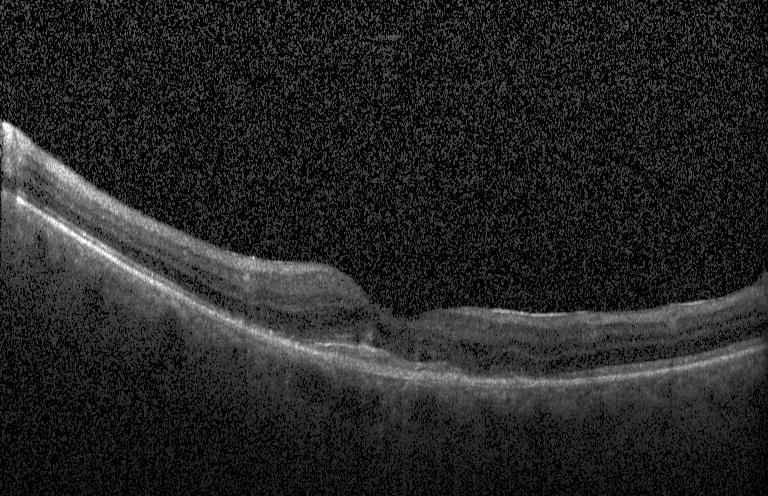
Finding: a choroidal neovascular membrane.